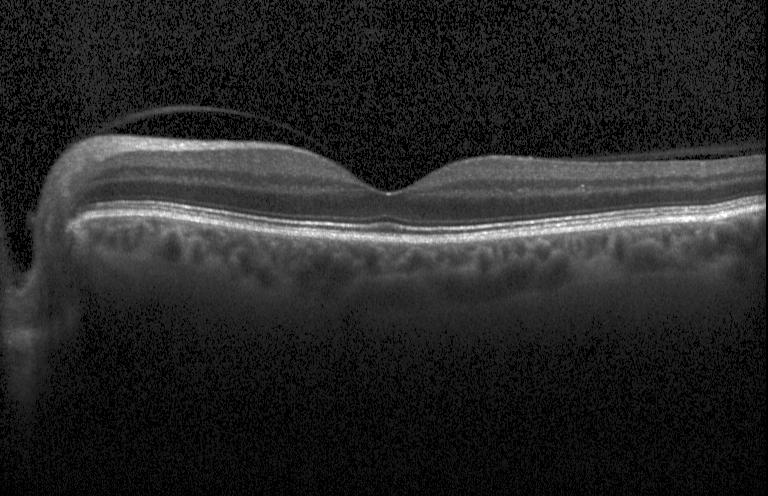
Horizontal scan through the fovea; retinal OCT cross-section; SD-OCT. Macular OCT: no evidence of choroidal neovascularization, diabetic macular edema, or drusen.